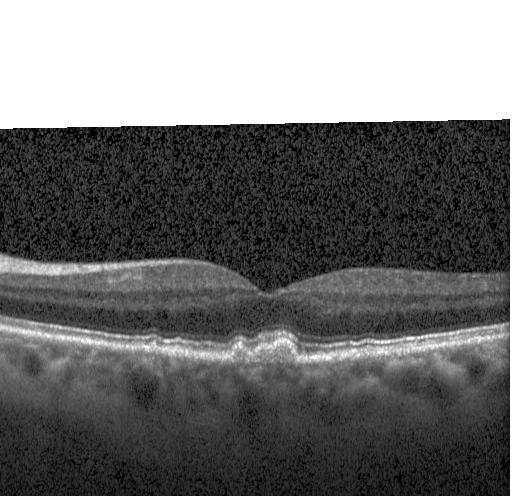 Macular scan. Spectral-domain OCT. Optical coherence tomography scan
Impression: multiple drusen.